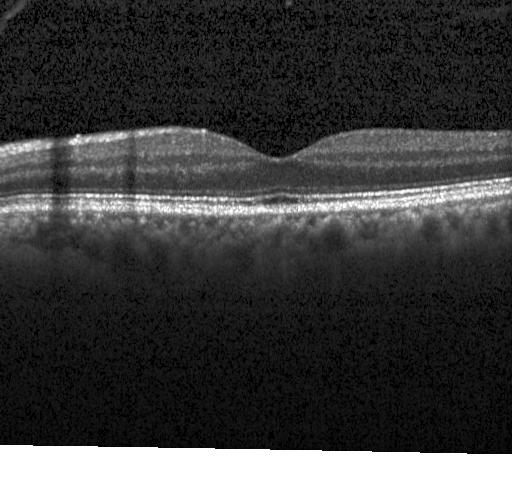

OCT B-scan showing no choroidal neovascularization, diabetic macular edema, or drusen.